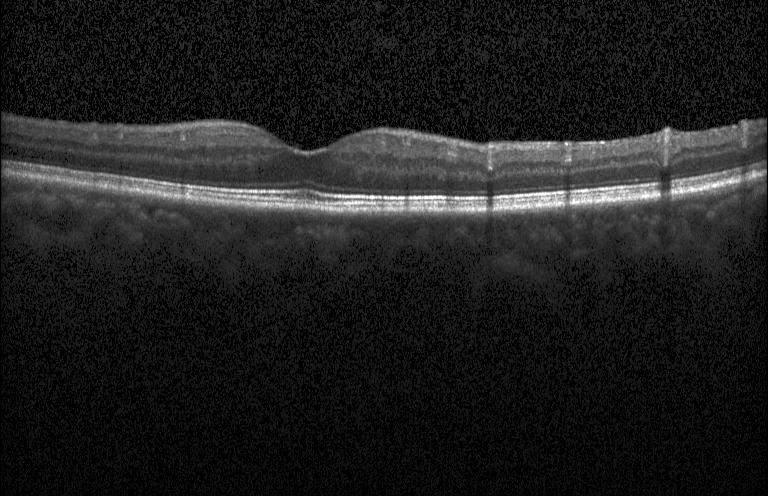
Diagnosis: no evidence of CNV, DME, or drusen.